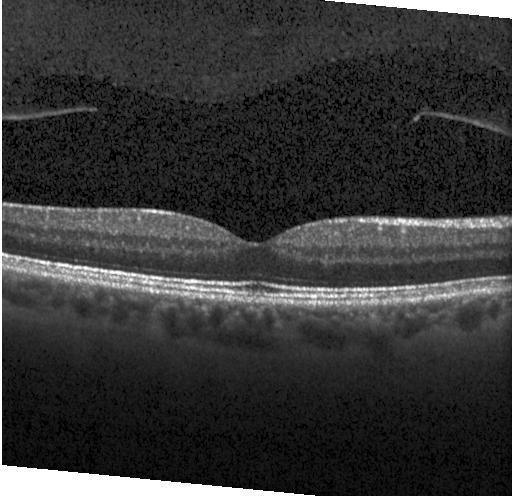

Retinal OCT B-scan. Heidelberg Spectralis OCT system. Centered on the fovea. Spectral-domain OCT
No evidence of CNV, DME, or drusen.